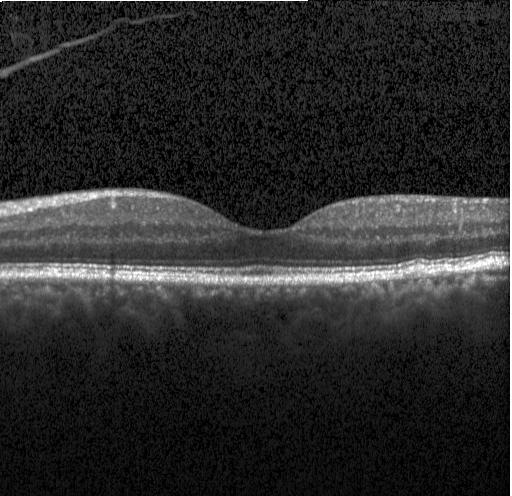

Retinal OCT B-scan.
Macular OCT: neither choroidal neovascularization, diabetic macular edema, nor drusen.